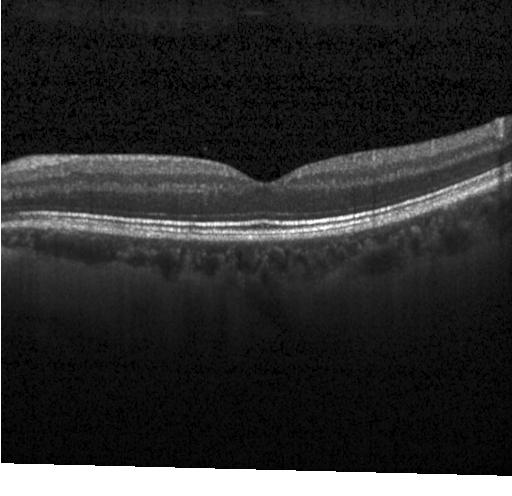 Optical coherence tomography B-scan — OCT finding: no choroidal neovascularization, no diabetic macular edema, and no drusen.